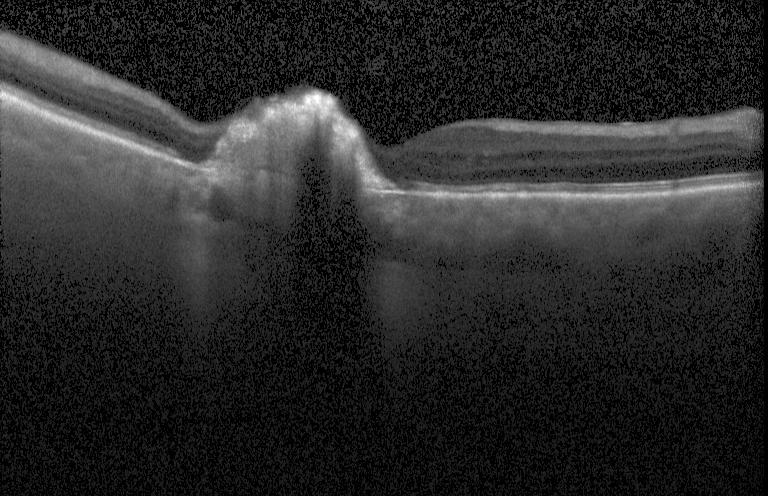 Acquired on a Heidelberg Spectralis · centered on the fovea · spectral-domain optical coherence tomography · retinal OCT B-scan. Impression: choroidal neovascularization.